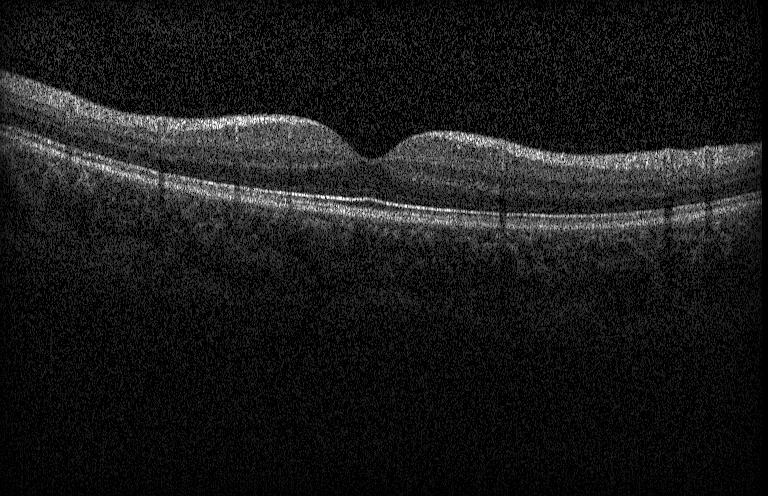
OCT B-scan showing no choroidal neovascularization, no diabetic macular edema, and no drusen.